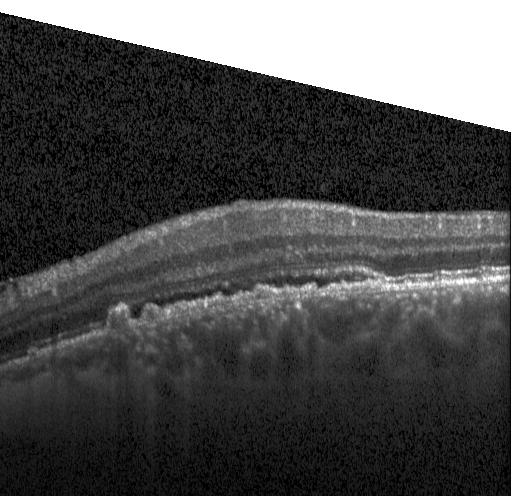
Retinal OCT cross-section. Macular scan. Heidelberg Spectralis.
Finding: CNV.